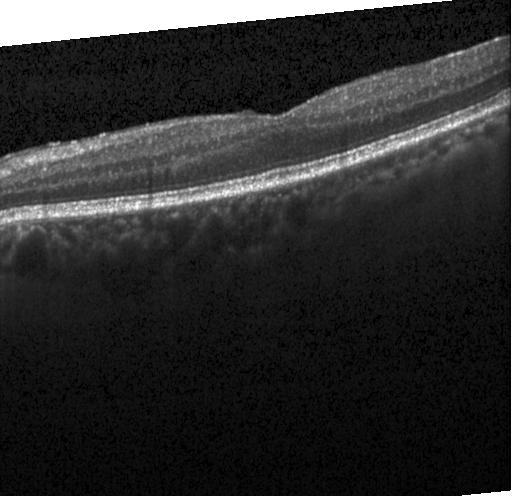

OCT scan showing no CNV, no DME, and no drusen.